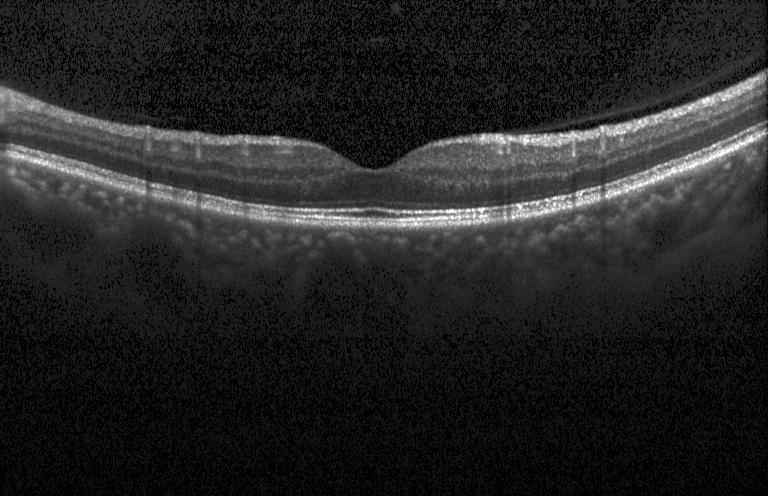 Retinal OCT cross-section showing no evidence of choroidal neovascularization, diabetic macular edema, or drusen.